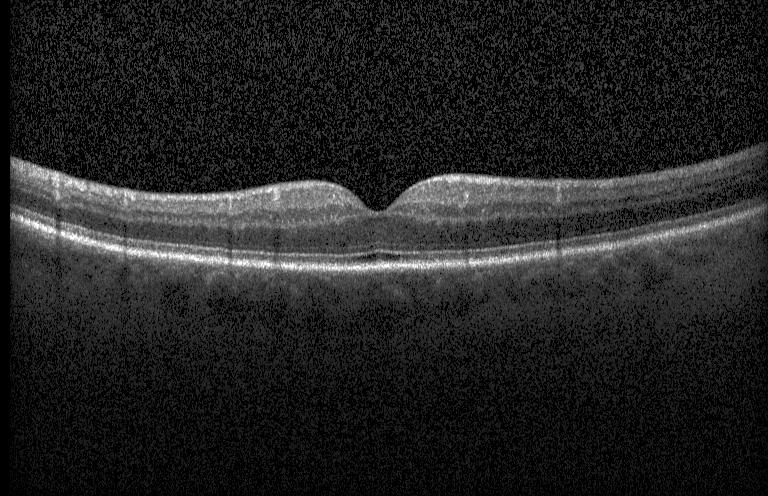 Diagnosis: neither choroidal neovascularization, diabetic macular edema, nor drusen.